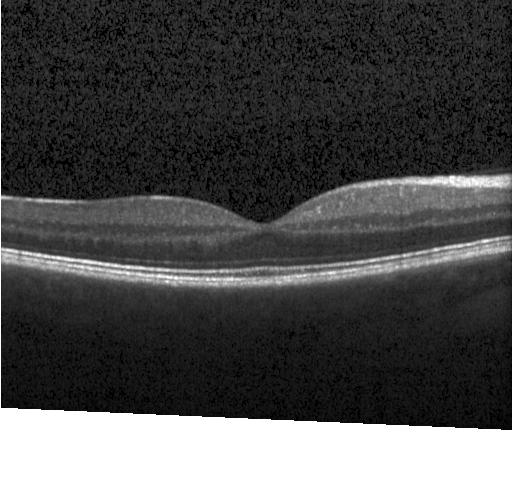

Heidelberg Spectralis OCT system · centered on the fovea · SD-OCT · optical coherence tomography B-scan. This B-scan demonstrates no evidence of choroidal neovascularization, diabetic macular edema, or drusen.